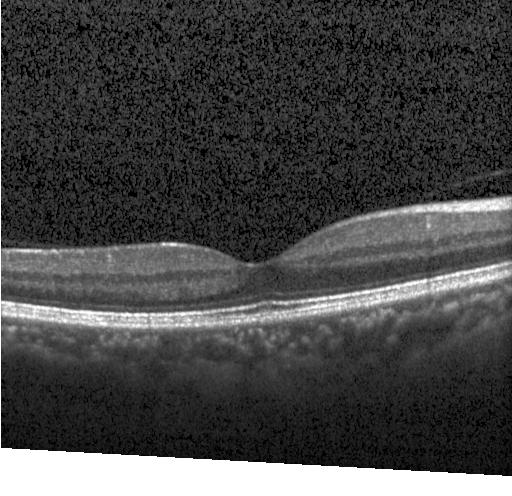
Impression: no CNV, DME, or drusen.